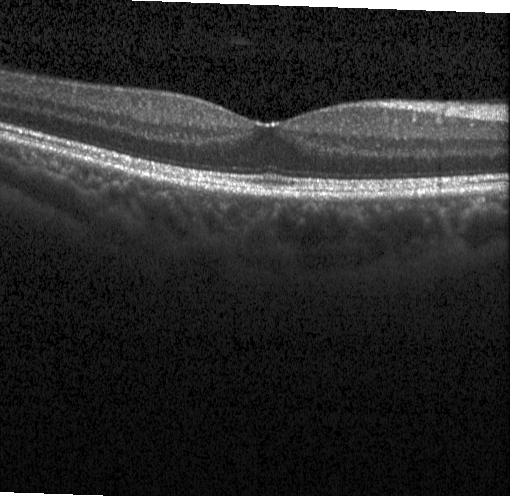 Horizontal scan through the fovea · retinal OCT B-scan. Assessment: neither CNV, DME, nor drusen.